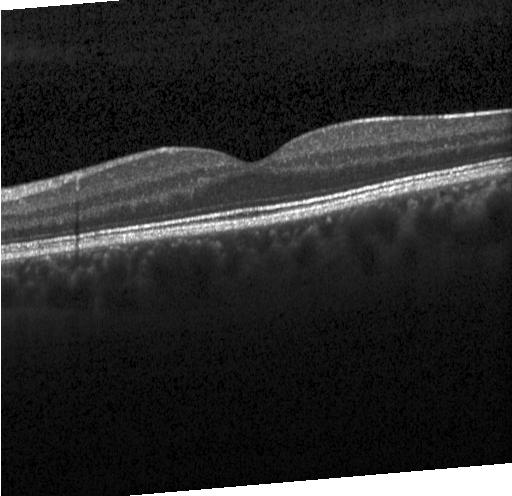

OCT B-scan showing no evidence of CNV, DME, or drusen.